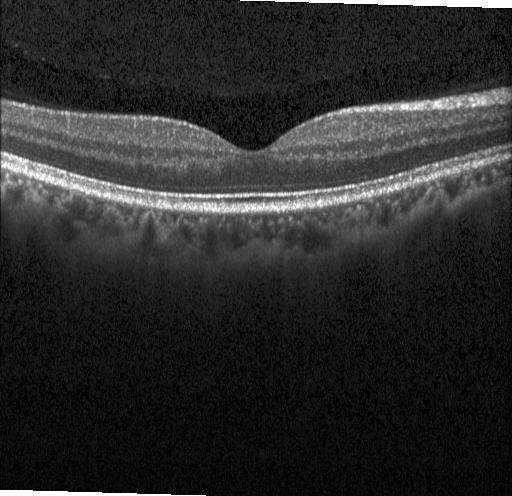 Heidelberg Spectralis, optical coherence tomography B-scan, horizontal scan through the fovea — Impression: no evidence of CNV, DME, or drusen.